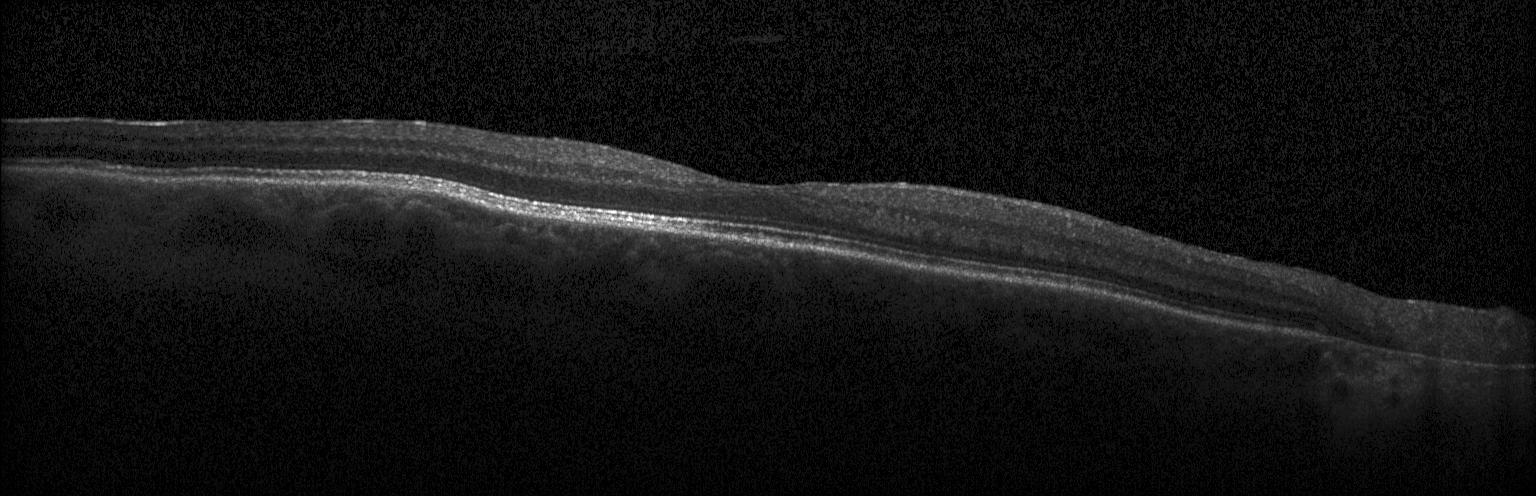
Dx: no evidence of choroidal neovascularization, diabetic macular edema, or drusen.